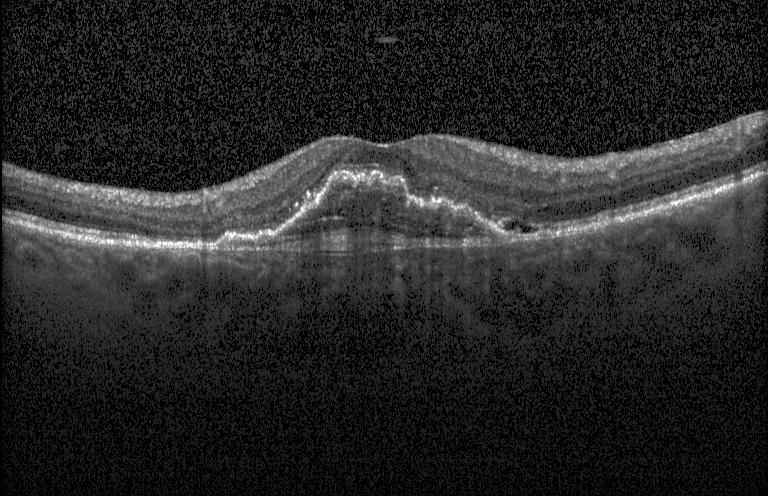

OCT line scan.
Impression: choroidal neovascularization (CNV).